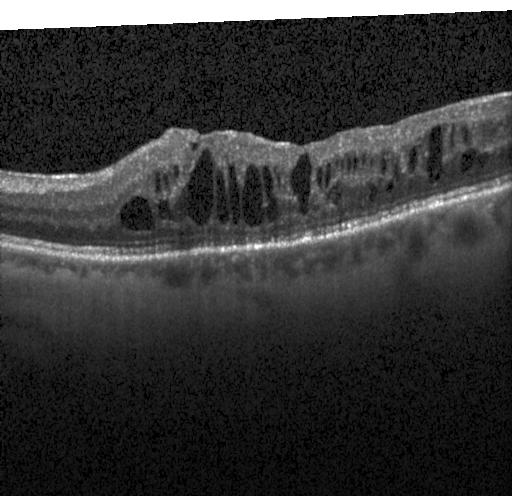 Finding: diabetic macular edema (DME).